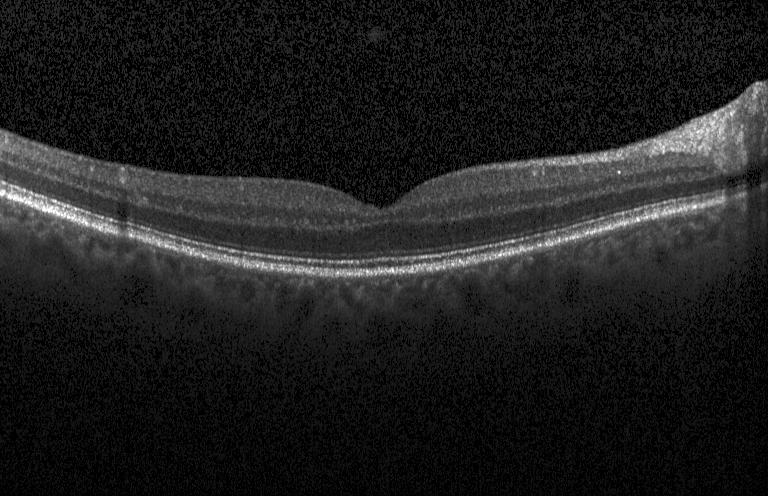

Optical coherence tomography scan — Finding: no choroidal neovascularization, no diabetic macular edema, and no drusen.